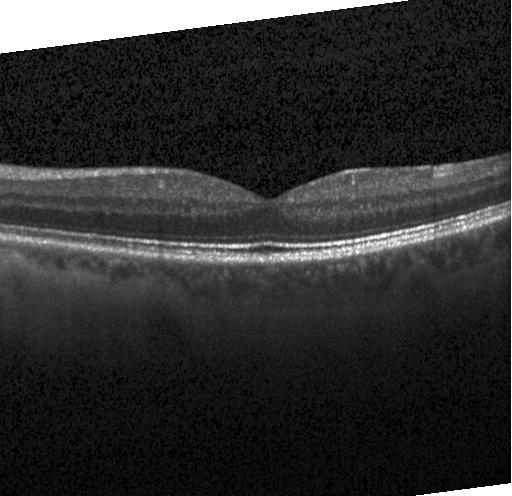
Retinal OCT cross-section · SD-OCT — This B-scan demonstrates no choroidal neovascularization, no diabetic macular edema, and no drusen.